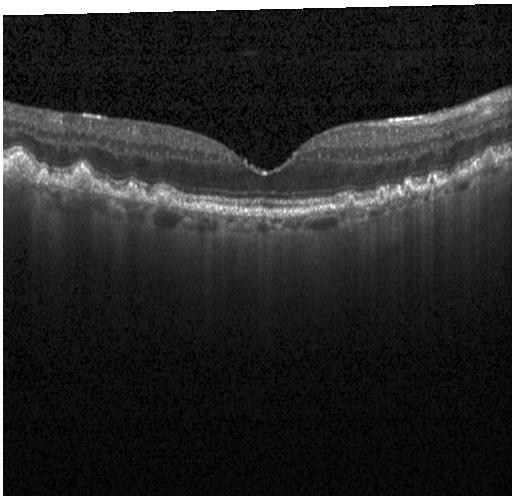
Instrument: Heidelberg Spectralis; SD-OCT; horizontal scan through the fovea; retinal OCT B-scan — Diagnosis: drusen.